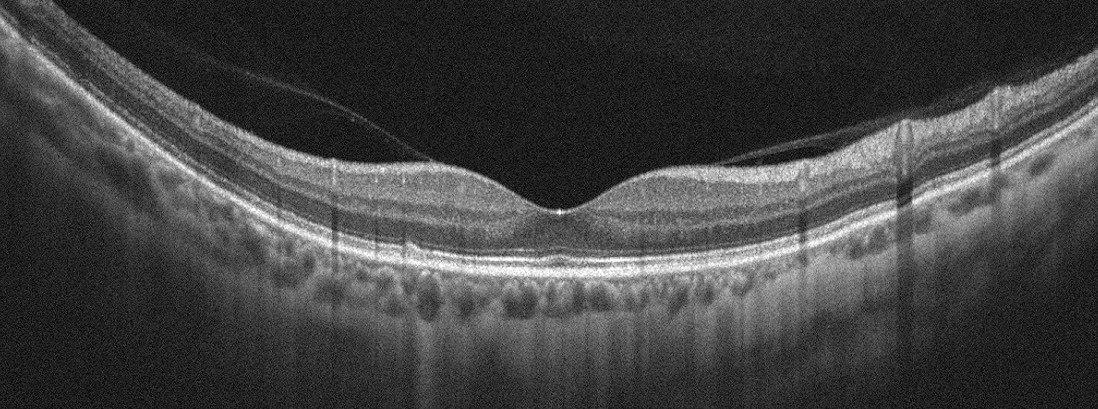
Impression: AMD.